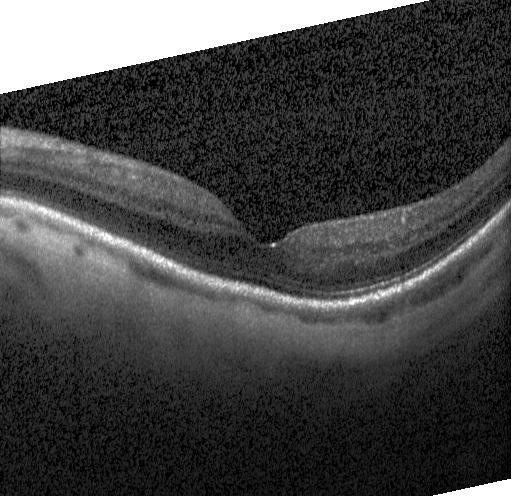 Optical coherence tomography scan
Assessment: no choroidal neovascularization, diabetic macular edema, or drusen.